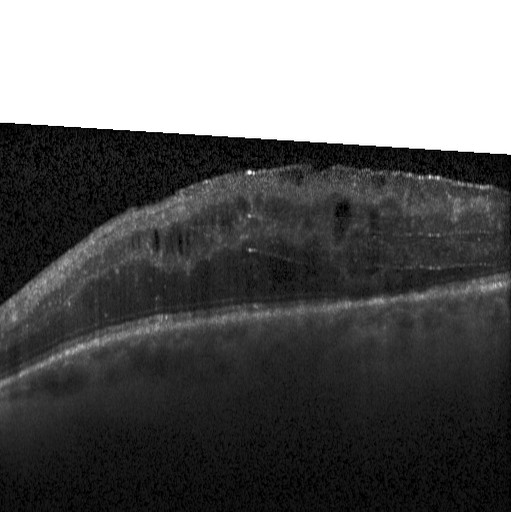

Heidelberg Spectralis, retinal OCT B-scan, spectral-domain OCT.
Assessment: diabetic macular edema.